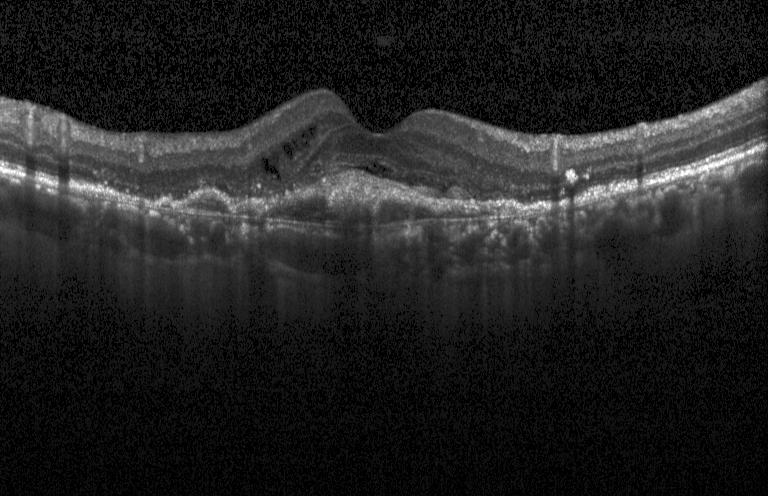
OCT B-scan. SD-OCT — Diagnosis: a choroidal neovascular membrane.